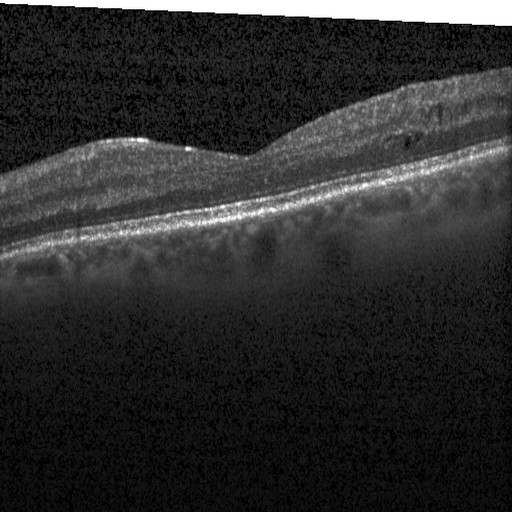
Diagnosis: DME.